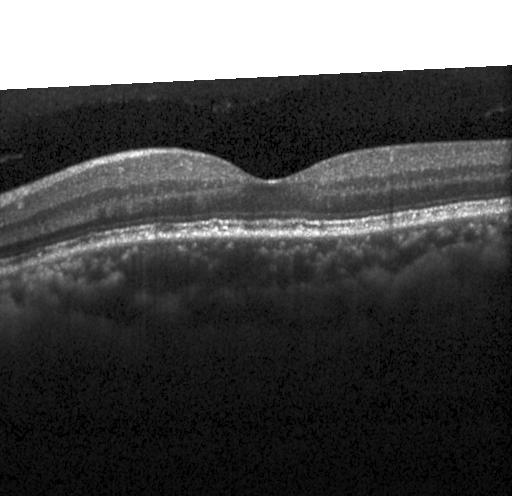 Optical coherence tomography B-scan
Assessment: multiple drusen.